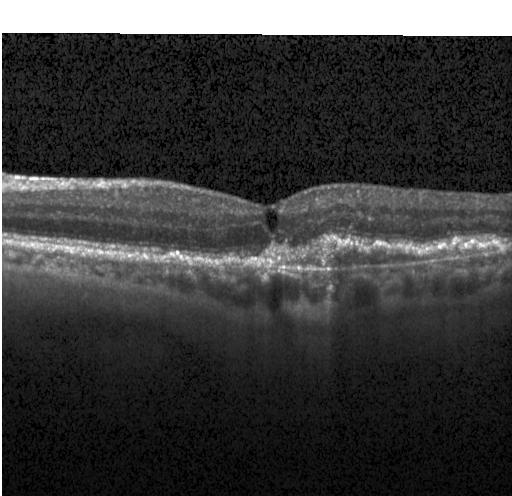

Retinal OCT cross-section; spectral-domain OCT — Diagnosis: a choroidal neovascular membrane.